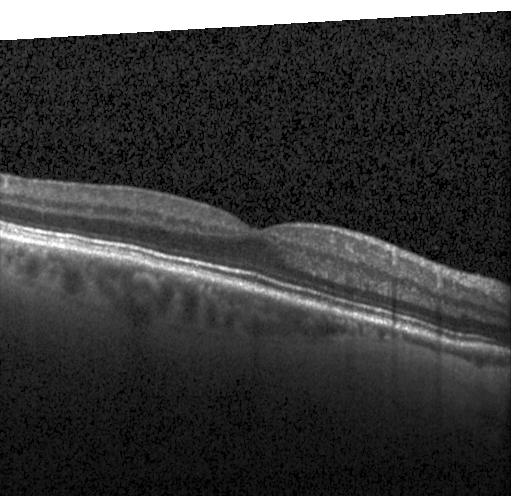
Impression: no choroidal neovascularization, no diabetic macular edema, and no drusen.